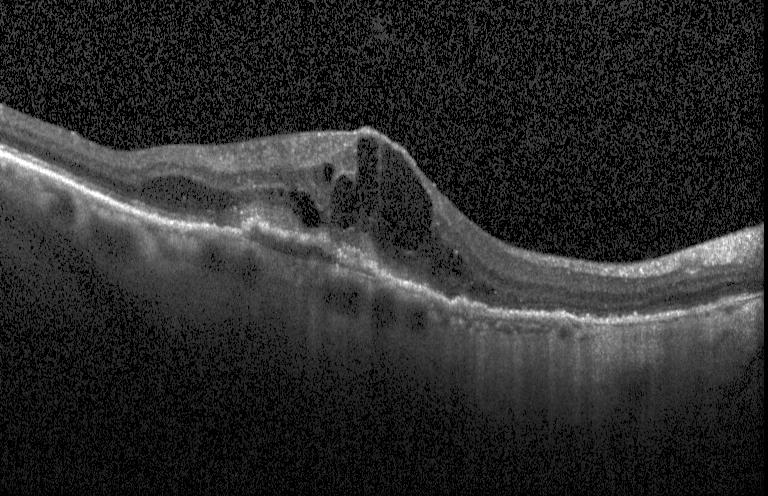

Retinal OCT B-scan; spectral-domain optical coherence tomography; Heidelberg Spectralis OCT system. Dx: CNV.